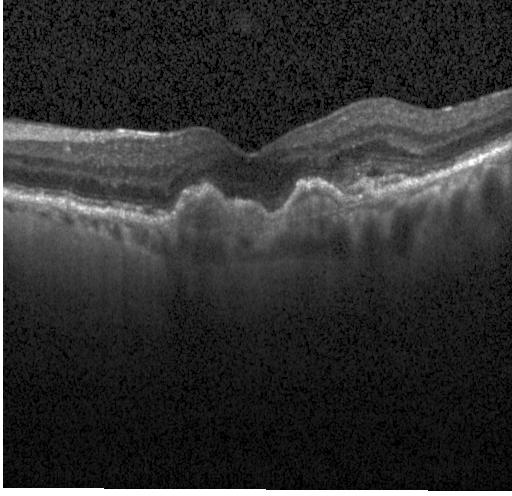 OCT B-scan; spectral-domain OCT; instrument: Heidelberg Spectralis.
This B-scan demonstrates a choroidal neovascular membrane.